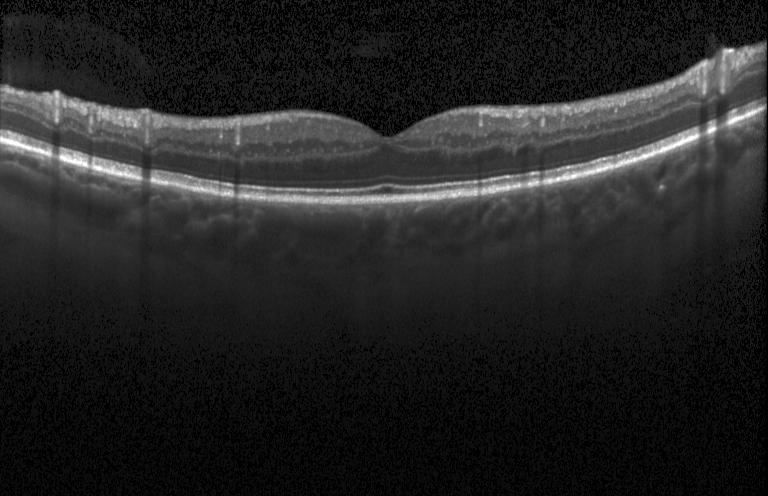
No choroidal neovascularization, no diabetic macular edema, and no drusen.